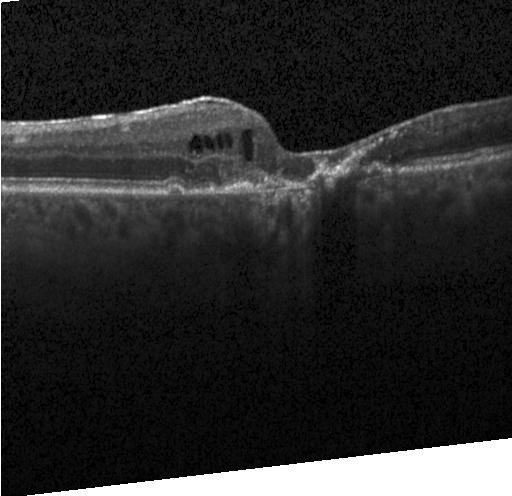

Finding: choroidal neovascularization.